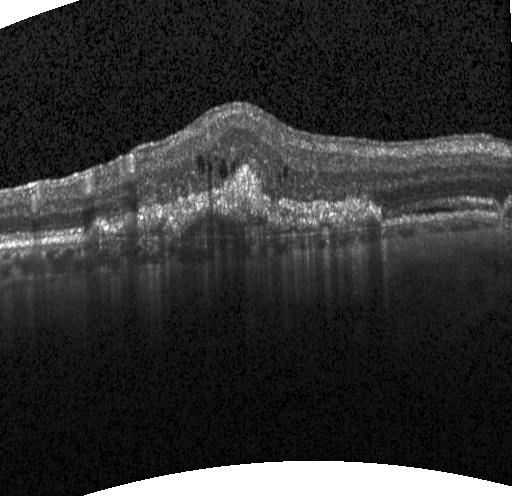 Spectral-domain OCT B-scan: CNV.